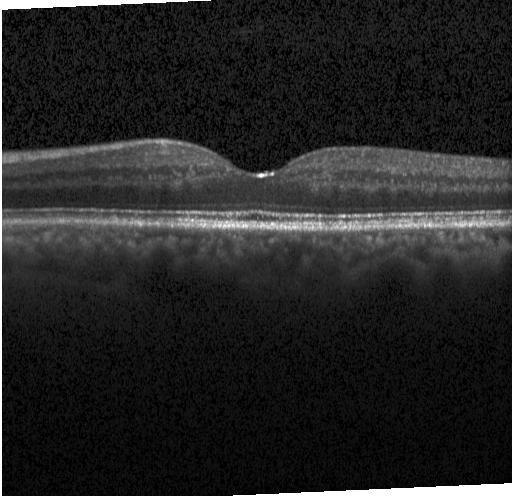
Through the macula, retinal OCT B-scan
Impression: no evidence of choroidal neovascularization, diabetic macular edema, or drusen.